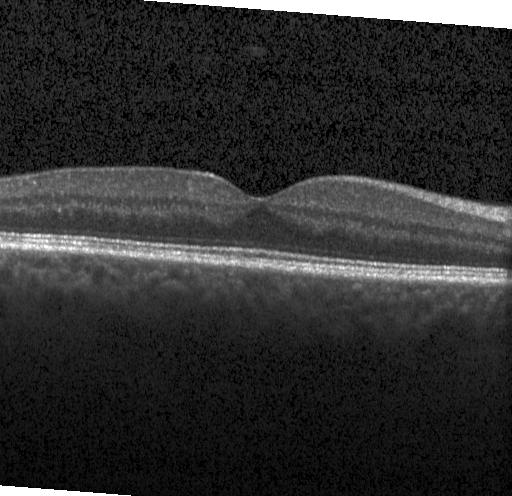

Retinal OCT B-scan. Instrument: Heidelberg Spectralis. Through the macula. Spectral-domain OCT.
This B-scan demonstrates no evidence of CNV, DME, or drusen.